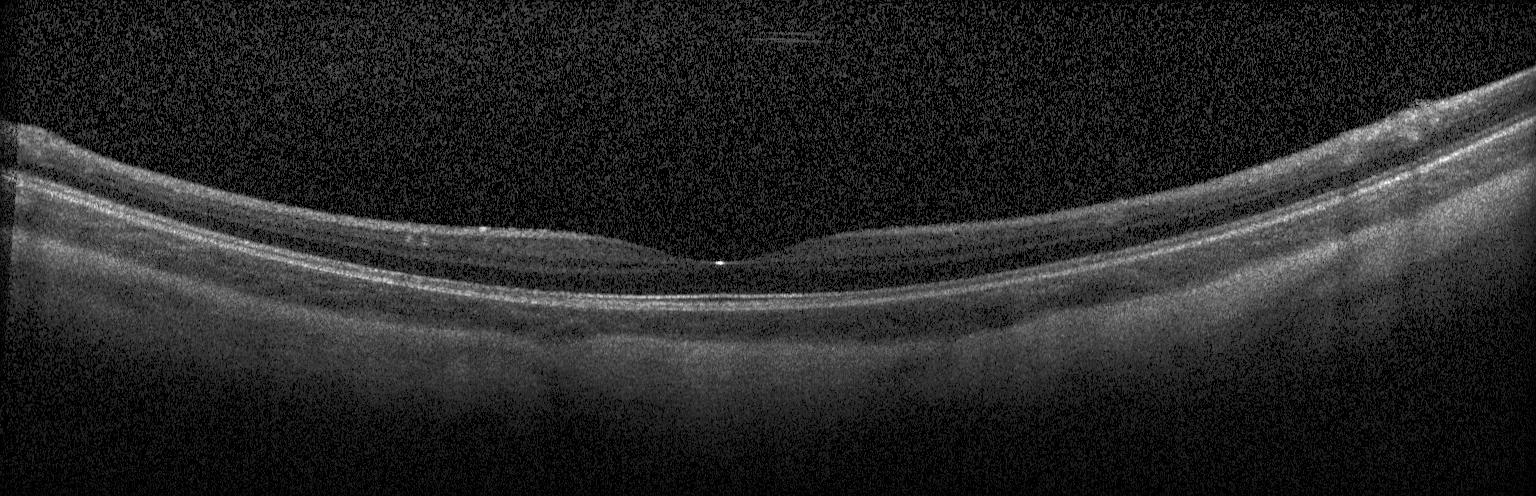
Through the macula, OCT line scan
Diagnosis: no evidence of choroidal neovascularization, diabetic macular edema, or drusen.